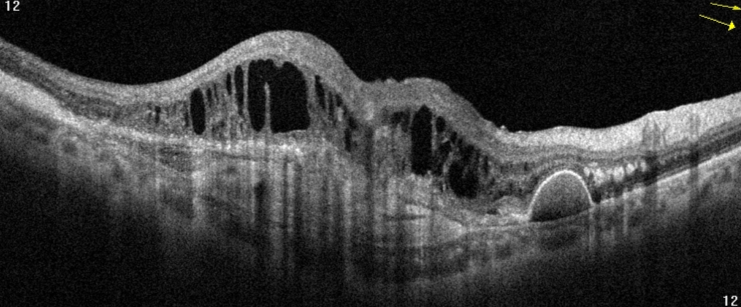
Acquired on an Optovue Avanti RTVue XR, retinal OCT cross-section, fovea-centered — Diagnosis: AMD.